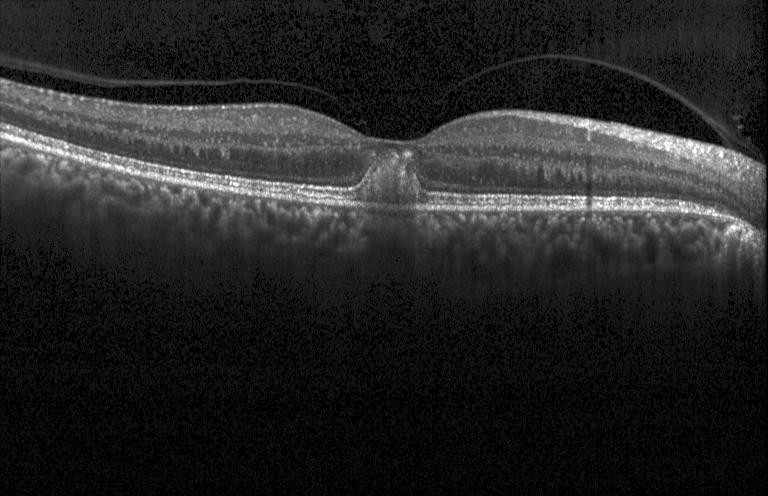
Optical coherence tomography B-scan
CNV.